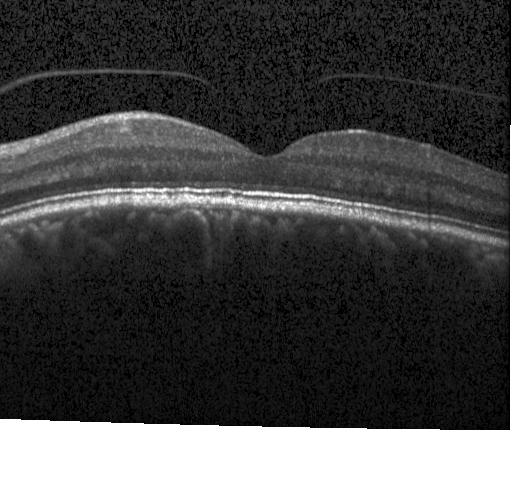
Retinal OCT B-scan.
OCT finding: no choroidal neovascularization, no diabetic macular edema, and no drusen.